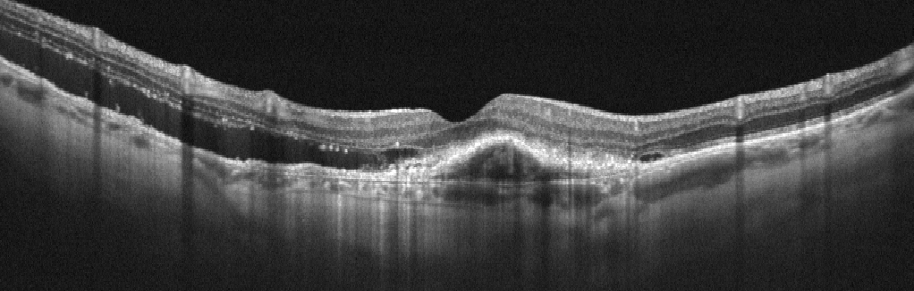 Through the macula, OCT B-scan, instrument: Optovue Avanti RTVue XR, oculus dexter. This B-scan demonstrates age-related macular degeneration (AMD).